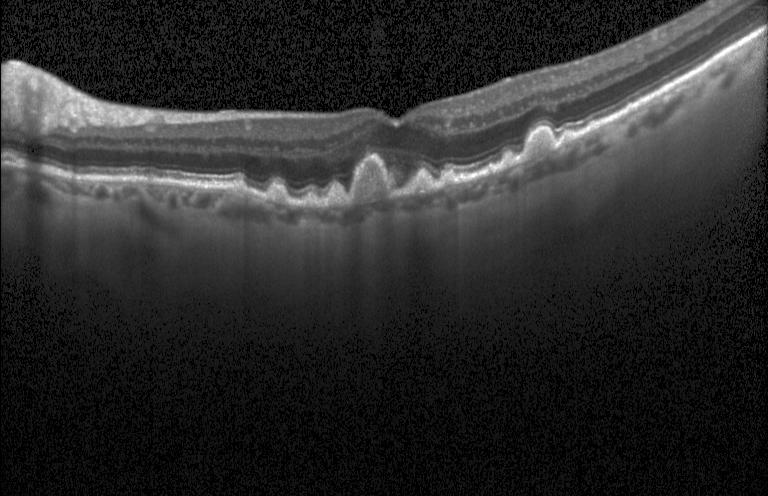

Optical coherence tomography scan · horizontal scan through the fovea · spectral-domain optical coherence tomography · Heidelberg Spectralis OCT system — The scan shows drusen.